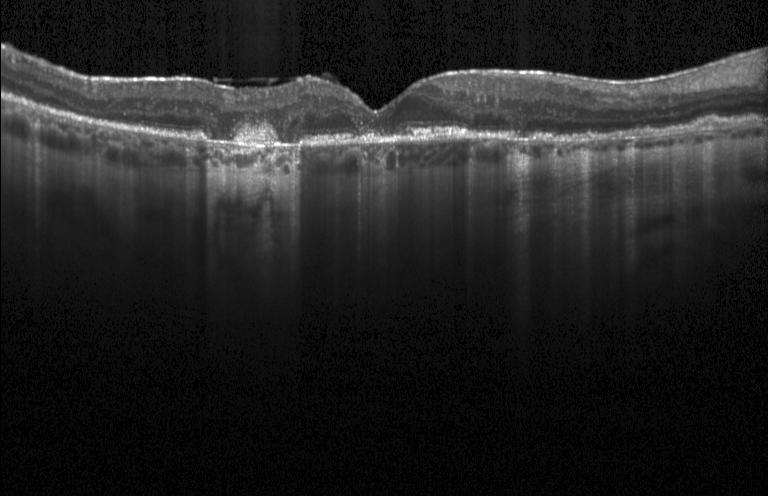
Impression: a choroidal neovascular membrane.